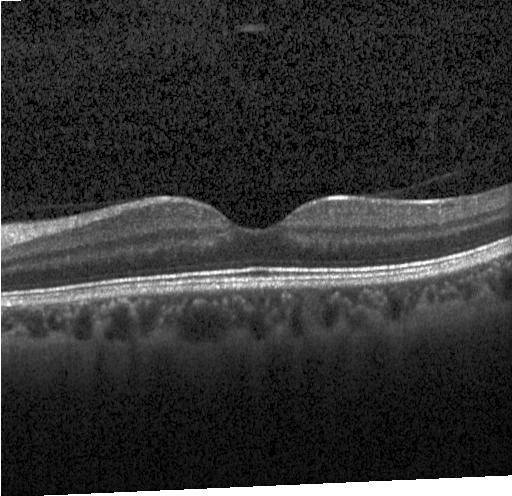 Diagnosis: no choroidal neovascularization, no diabetic macular edema, and no drusen.